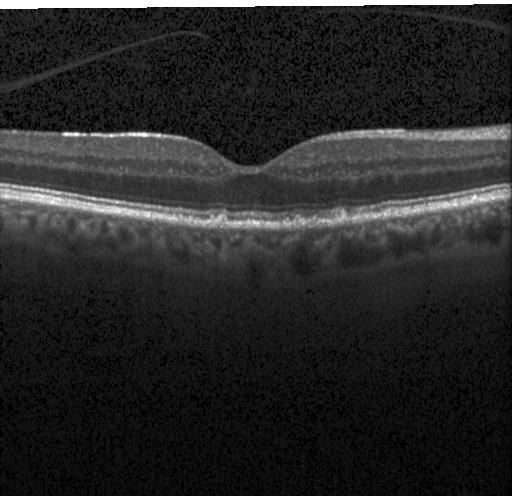
Instrument: Heidelberg Spectralis, spectral-domain optical coherence tomography, optical coherence tomography B-scan. This B-scan demonstrates drusen.